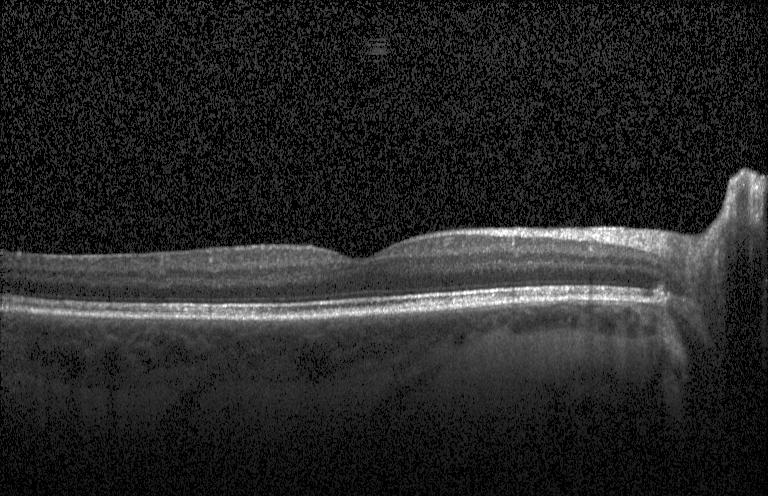 Optical coherence tomography B-scan.
Finding: neither CNV, DME, nor drusen.